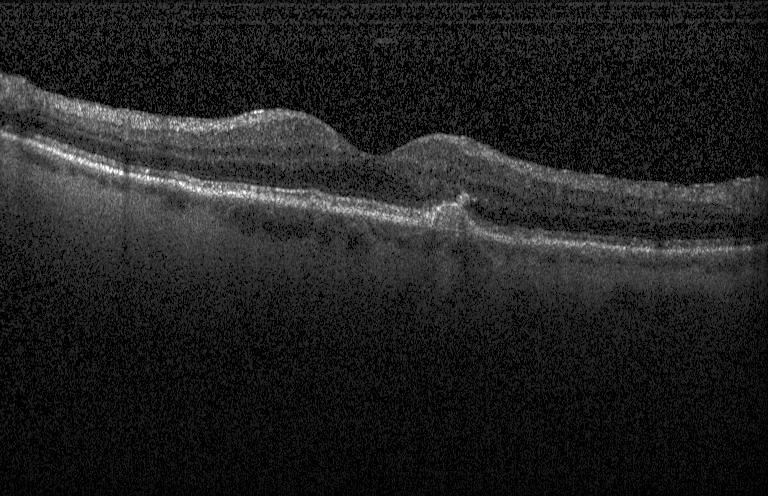

Finding: multiple drusen.